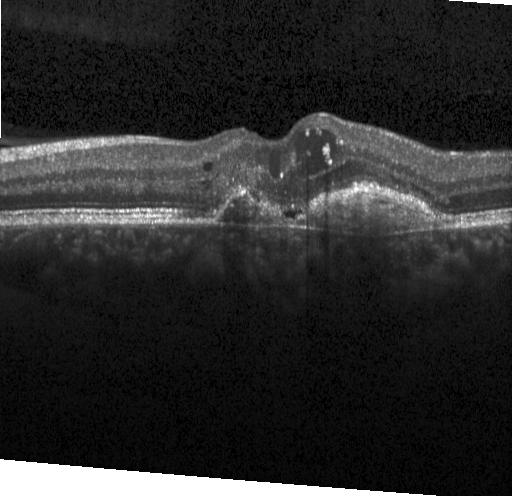
Optical coherence tomography scan; centered on the fovea; spectral-domain OCT; acquired on a Heidelberg Spectralis. This B-scan demonstrates a choroidal neovascular membrane.